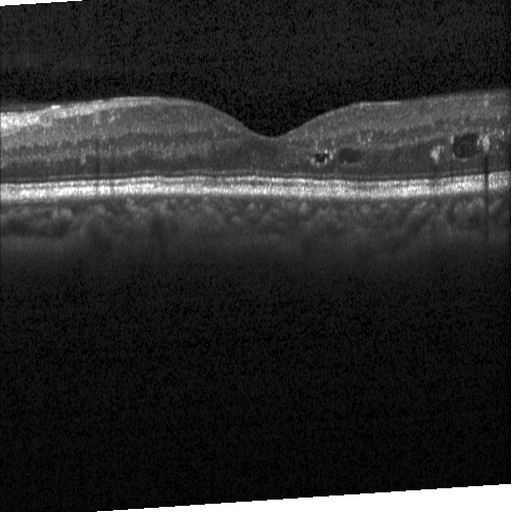 Dx: DME.